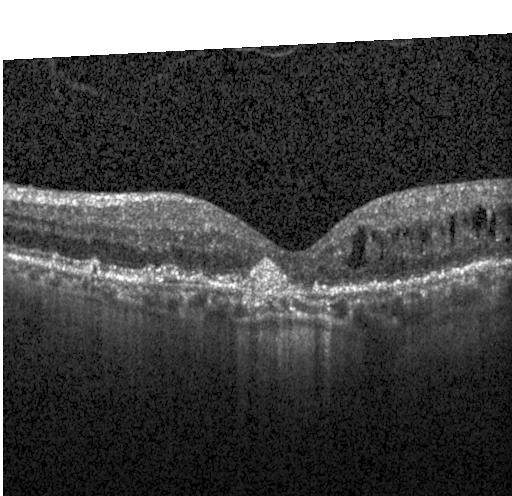
OCT line scan · instrument: Heidelberg Spectralis.
Diagnosis: choroidal neovascularization.